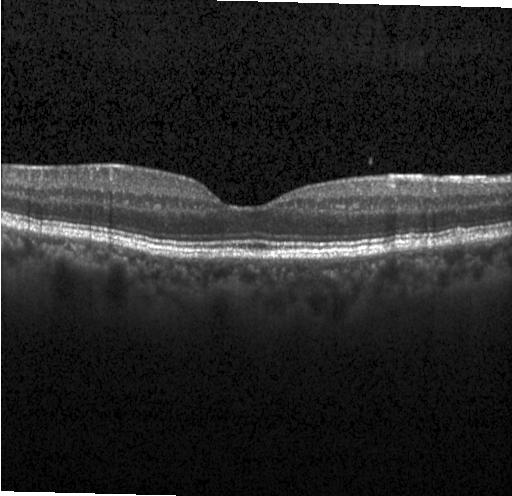

Finding: no evidence of choroidal neovascularization, diabetic macular edema, or drusen.